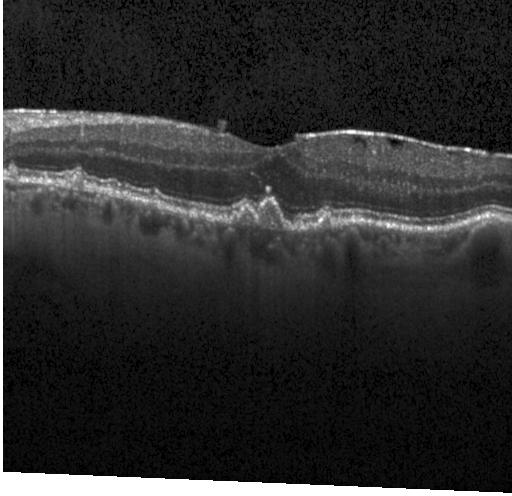 Diagnosis: drusen.